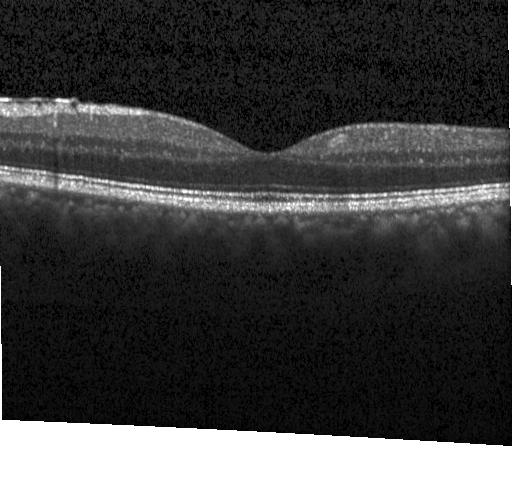

Through the macula; spectral-domain OCT; OCT B-scan — Diagnosis: no evidence of CNV, DME, or drusen.